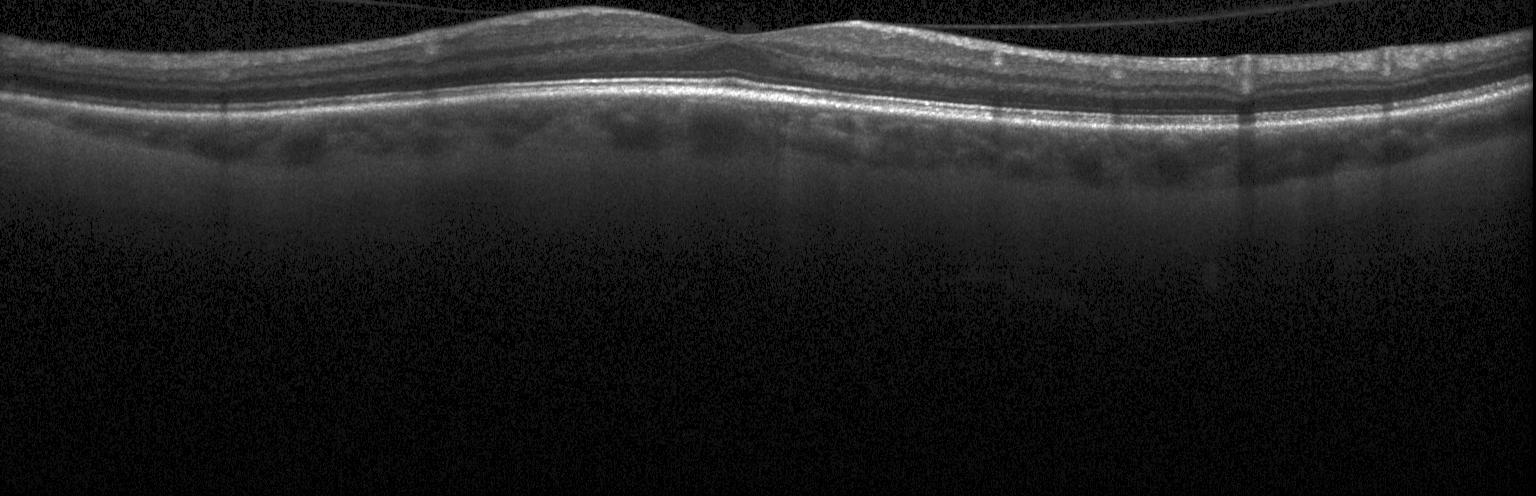
SD-OCT; retinal OCT cross-section
The scan shows no evidence of CNV, DME, or drusen.